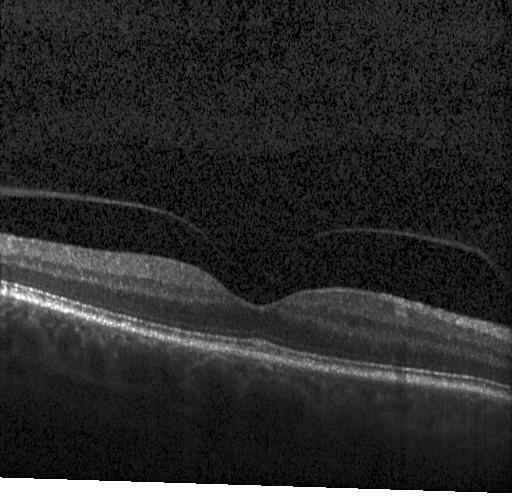

Optical coherence tomography scan. Spectral-domain OCT. Centered on the fovea. Heidelberg Spectralis
Macular OCT: no CNV, DME, or drusen.